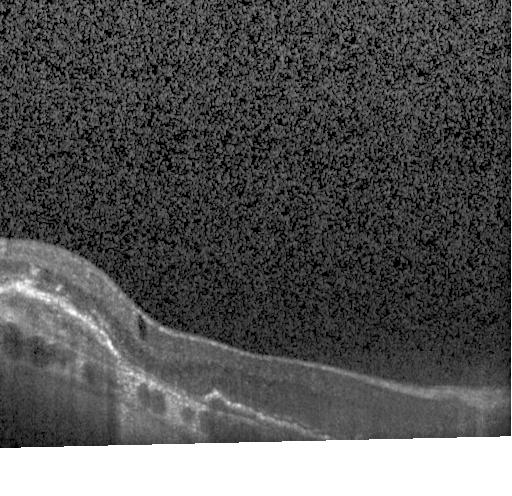
Optical coherence tomography scan — Macular OCT: choroidal neovascularization.